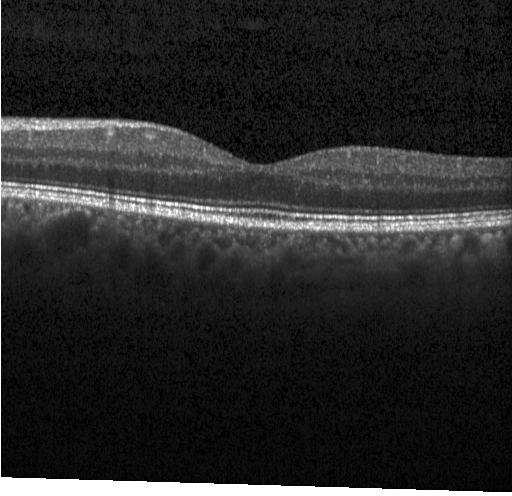 SD-OCT. Retinal OCT B-scan. Macular scan. Instrument: Heidelberg Spectralis — OCT finding: no choroidal neovascularization, no diabetic macular edema, and no drusen.